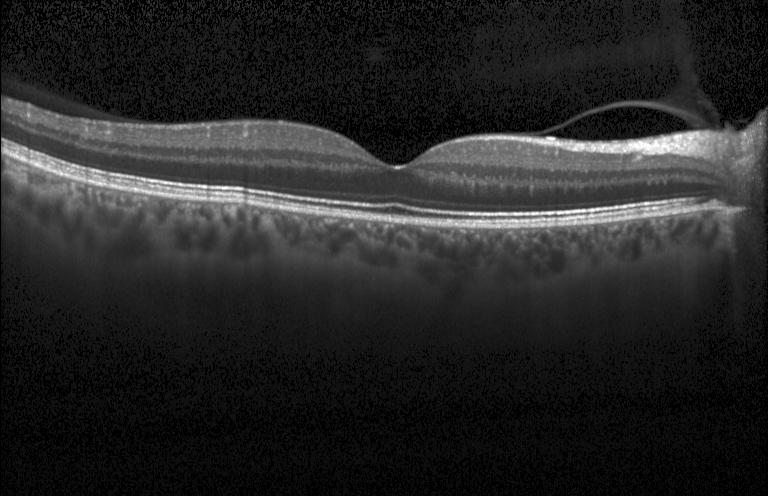
Optical coherence tomography scan. Finding: no choroidal neovascularization, no diabetic macular edema, and no drusen.